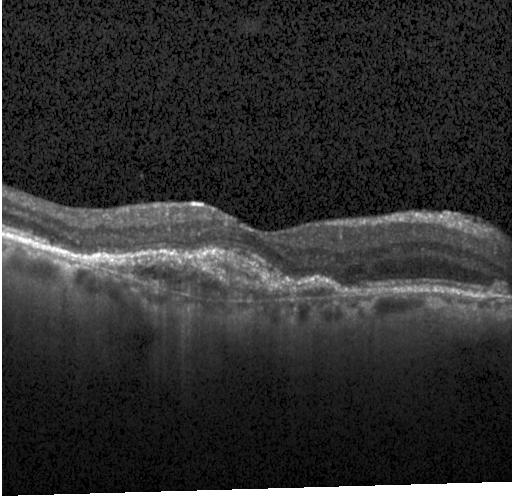 Impression: choroidal neovascularization (CNV).